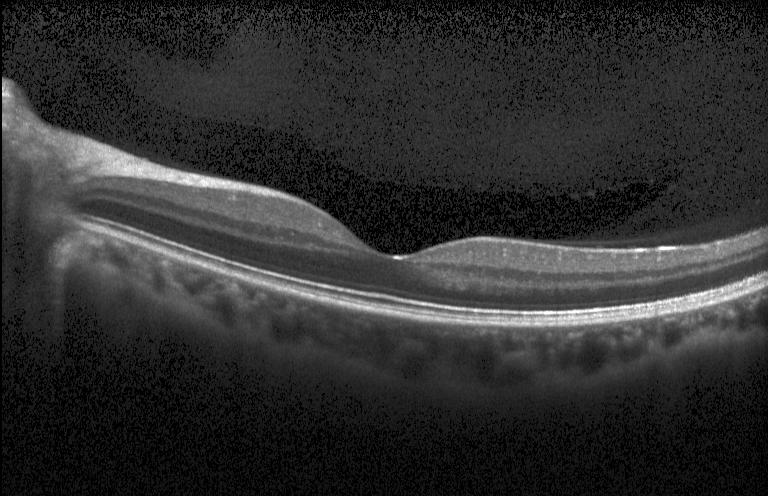 Optical coherence tomography B-scan. Heidelberg Spectralis OCT system — Diagnosis: no evidence of choroidal neovascularization, diabetic macular edema, or drusen.